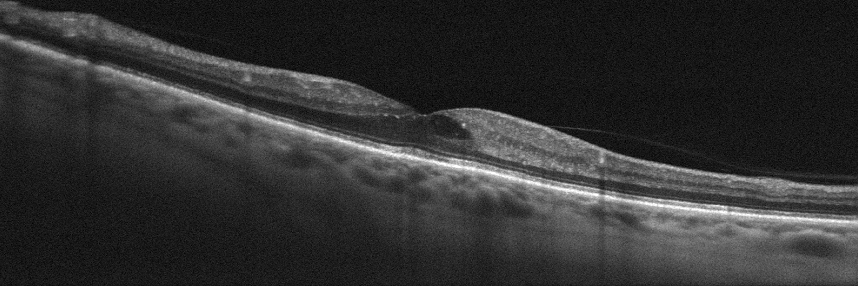
Acquired on an Optovue Avanti RTVue XR · OCT B-scan — Diabetic macular edema.